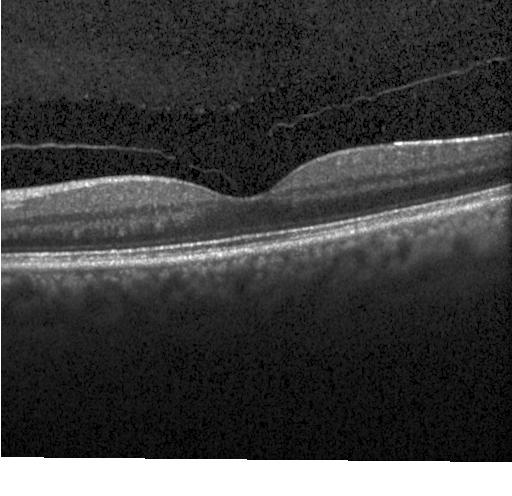 OCT line scan · macular scan — OCT finding: no choroidal neovascularization, no diabetic macular edema, and no drusen.